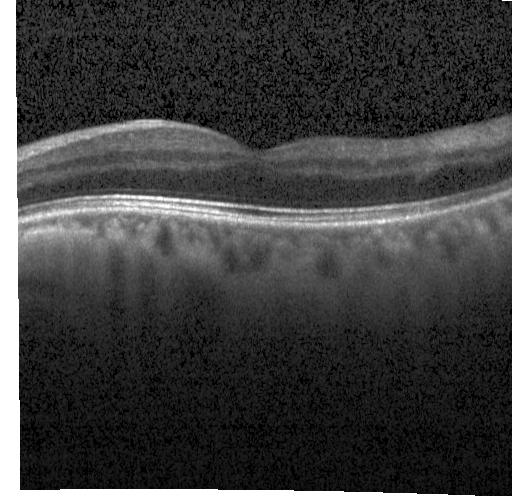

Instrument: Heidelberg Spectralis, through the macula, spectral-domain OCT, OCT B-scan.
Finding: no evidence of choroidal neovascularization, diabetic macular edema, or drusen.